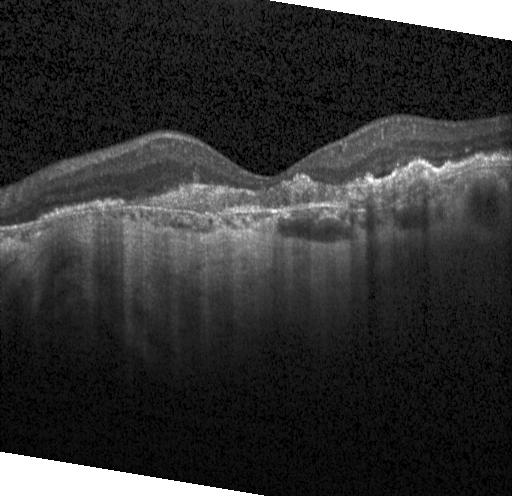

Retinal OCT cross-section; spectral-domain OCT; through the macula; Heidelberg Spectralis OCT system.
Macular OCT: choroidal neovascularization (CNV).